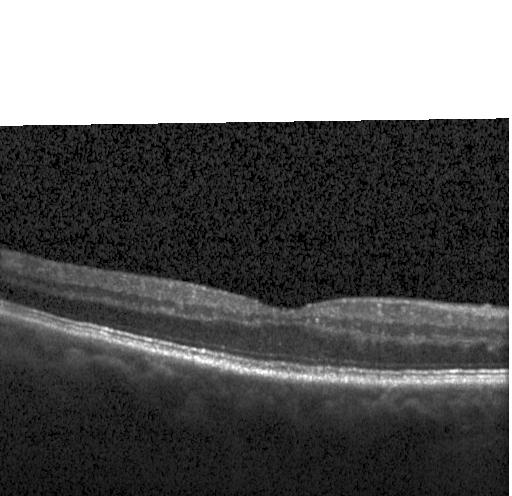 Macular scan. Optical coherence tomography B-scan.
Assessment: no choroidal neovascularization, no diabetic macular edema, and no drusen.